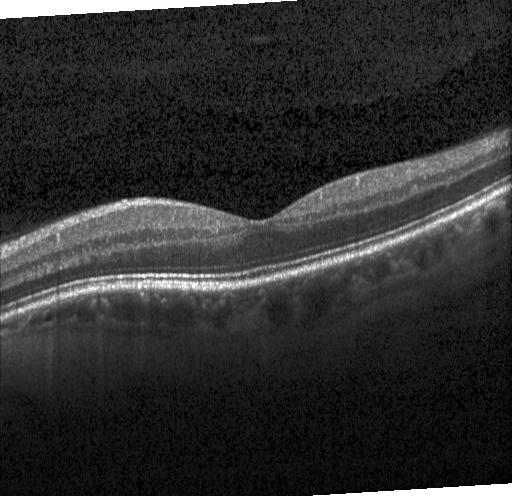
Instrument: Heidelberg Spectralis. OCT B-scan. Centered on the fovea
This B-scan demonstrates no choroidal neovascularization, diabetic macular edema, or drusen.